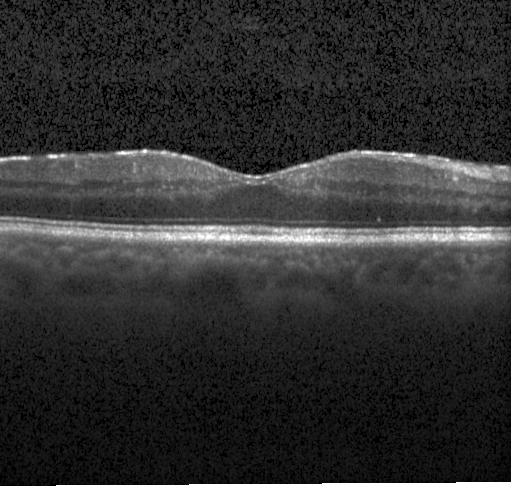 OCT scan showing no choroidal neovascularization, no diabetic macular edema, and no drusen.